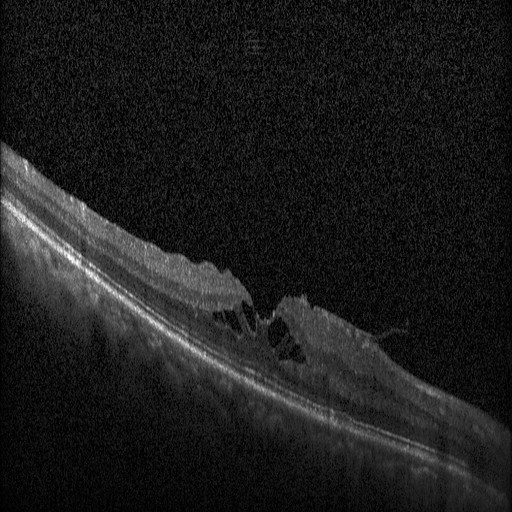

OCT B-scan showing diabetic macular edema (DME).